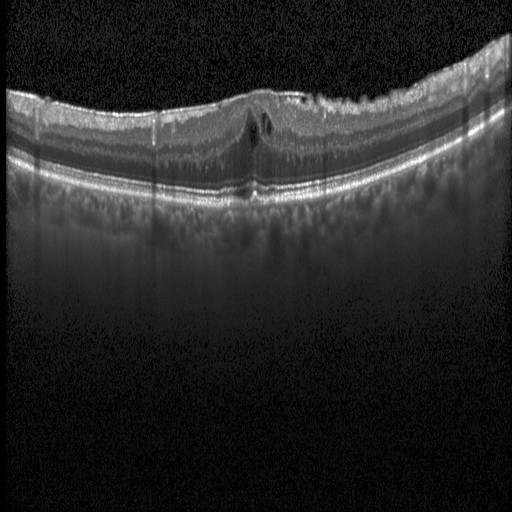

Fovea-centered. Optical coherence tomography scan. Heidelberg Spectralis
This B-scan demonstrates DME.